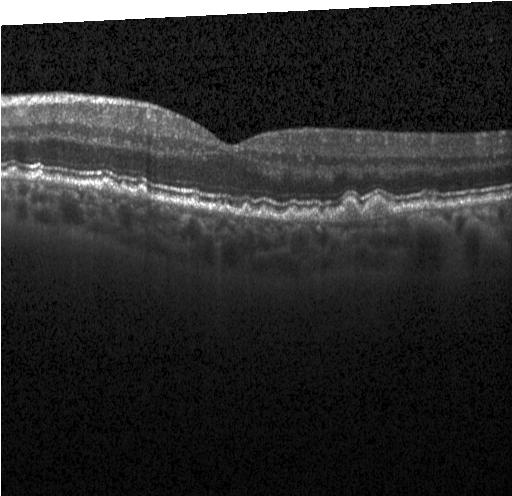
SD-OCT. Through the macula. Optical coherence tomography B-scan
Dx: sub-RPE drusenoid deposits.